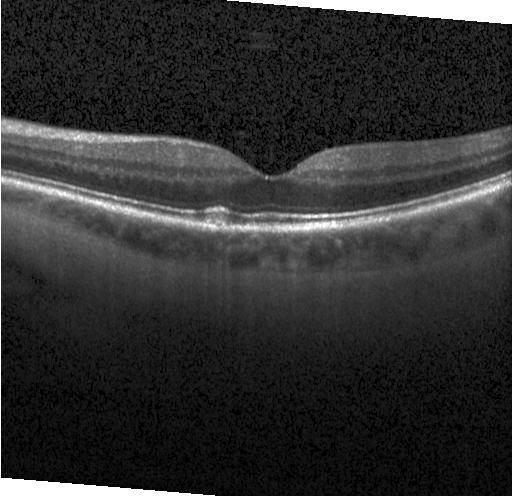 Neither CNV, DME, nor drusen.